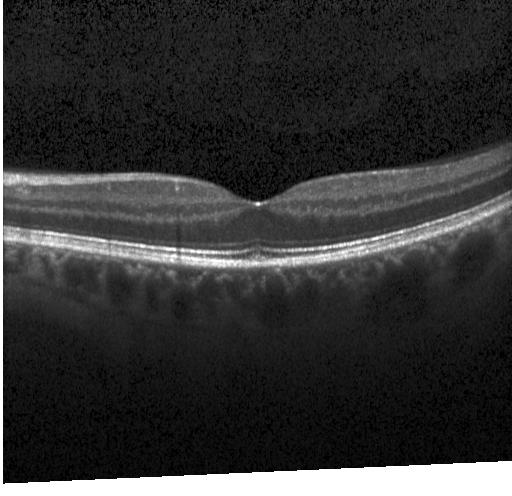 Retinal OCT B-scan.
Finding: no choroidal neovascularization, diabetic macular edema, or drusen.